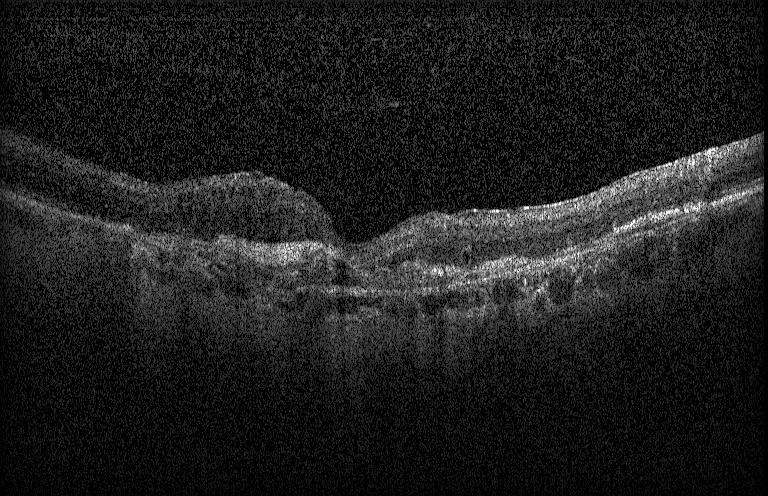
Diagnosis: choroidal neovascularization.